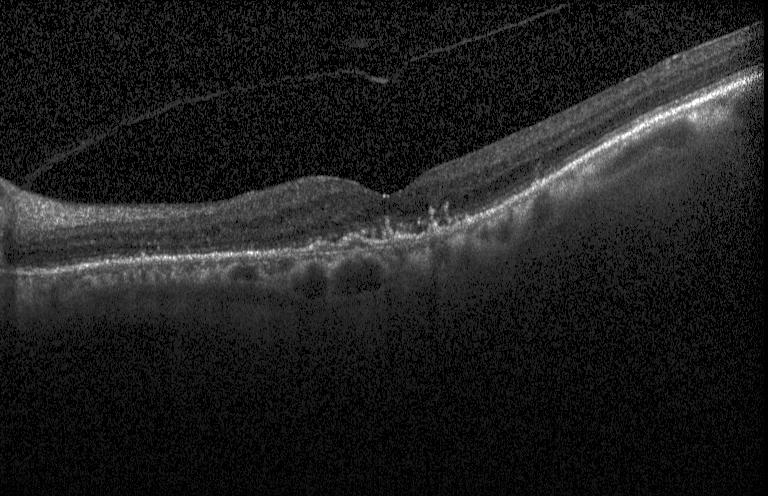

A choroidal neovascular membrane.